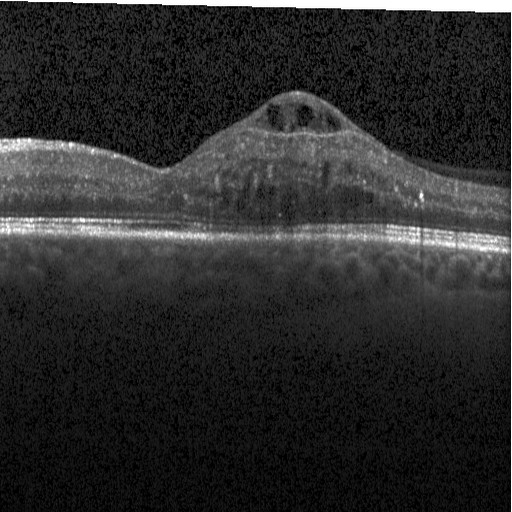 Centered on the fovea · optical coherence tomography B-scan · SD-OCT · Heidelberg Spectralis OCT system.
The scan shows DME.